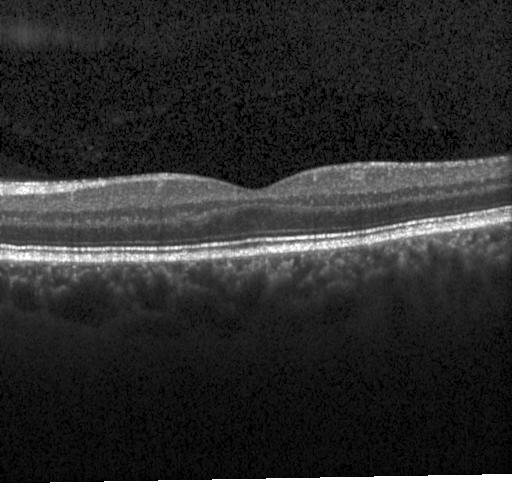 OCT B-scan showing neither choroidal neovascularization, diabetic macular edema, nor drusen.